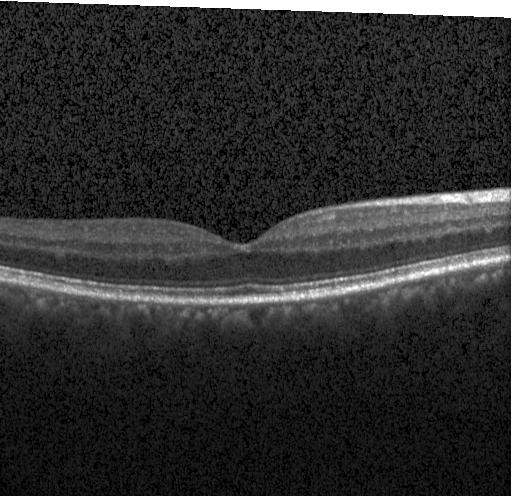
This B-scan demonstrates no choroidal neovascularization, diabetic macular edema, or drusen.